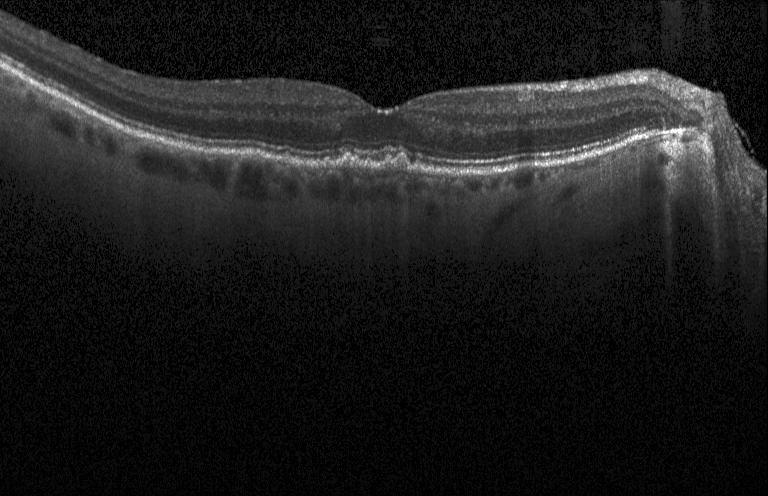

Spectral-domain optical coherence tomography. OCT line scan. Assessment: drusen.